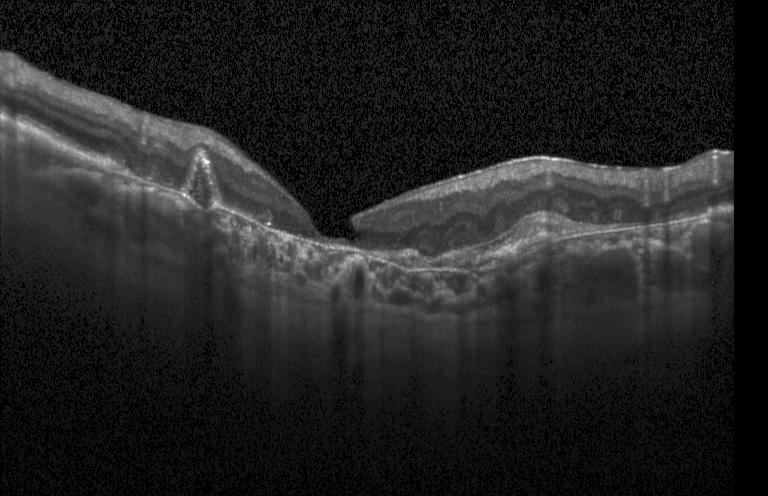

Retinal OCT cross-section — A choroidal neovascular membrane.